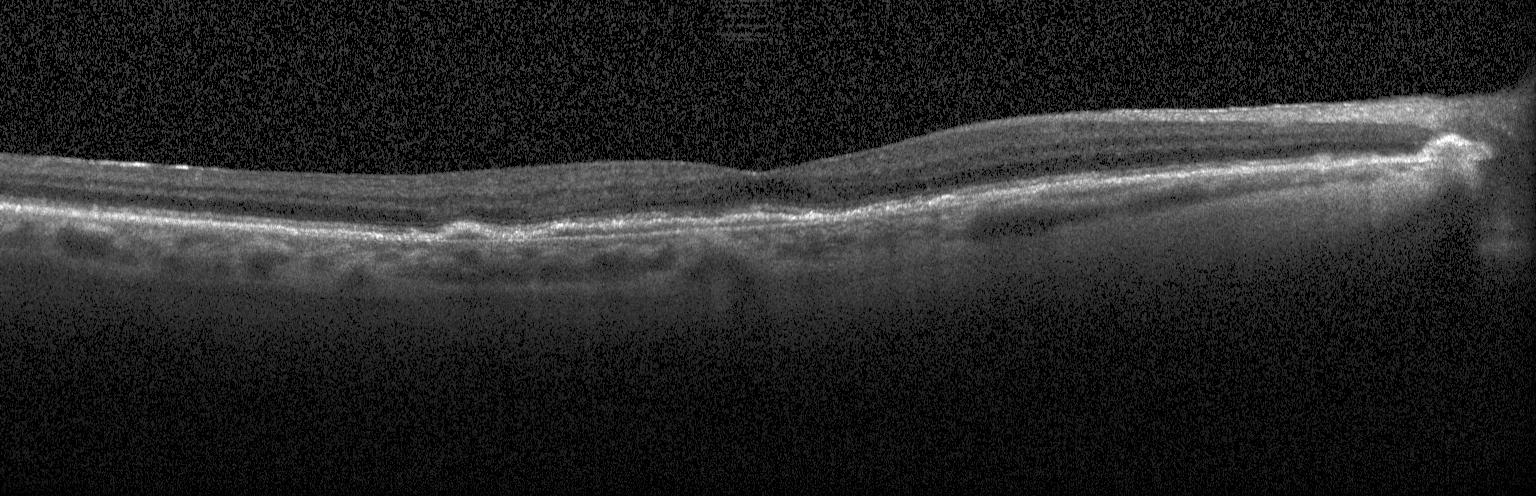

SD-OCT; optical coherence tomography scan; Heidelberg Spectralis — The scan shows CNV.